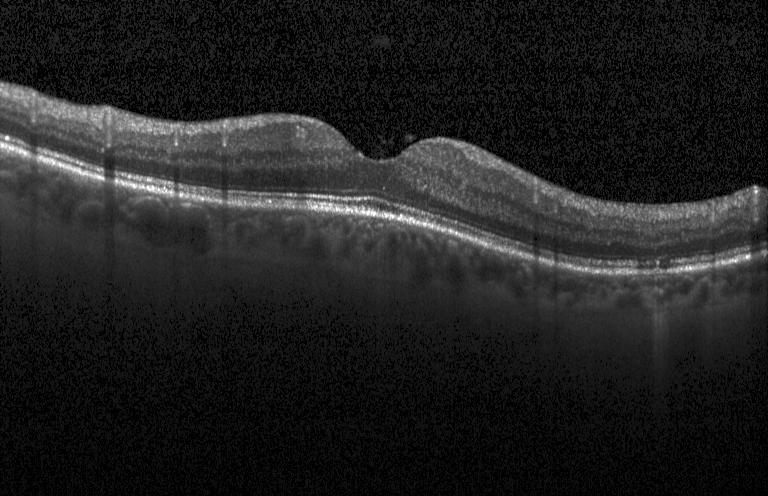
Optical coherence tomography scan — No choroidal neovascularization, no diabetic macular edema, and no drusen.